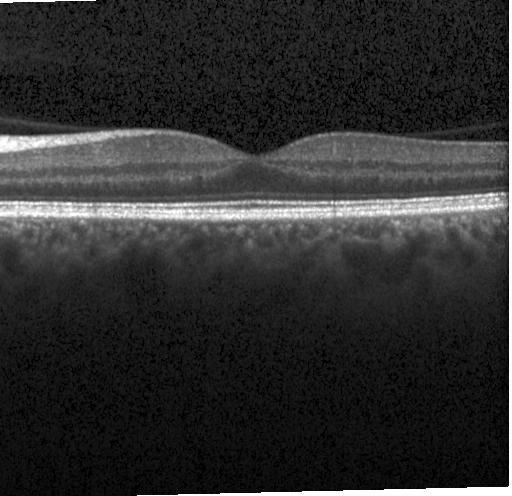

Retinal OCT B-scan. Heidelberg Spectralis. Through the macula.
Impression: no choroidal neovascularization, diabetic macular edema, or drusen.